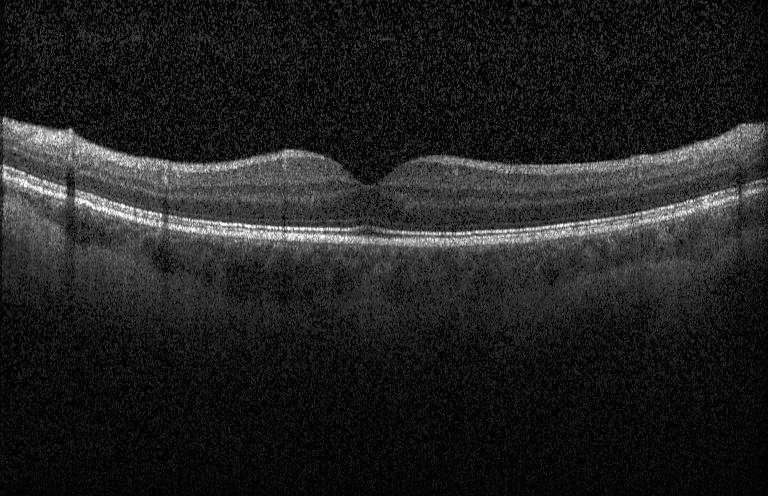 OCT finding: no choroidal neovascularization, diabetic macular edema, or drusen.